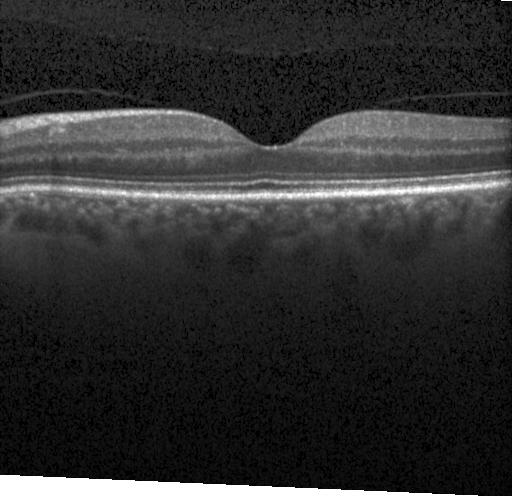

SD-OCT · retinal OCT cross-section.
Diagnosis: no choroidal neovascularization, no diabetic macular edema, and no drusen.